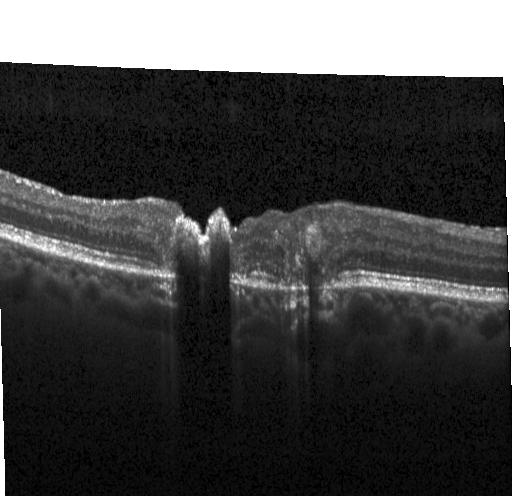

OCT B-scan showing choroidal neovascularization (CNV).